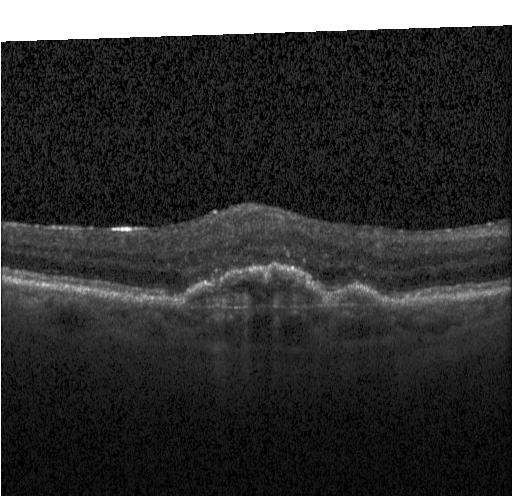

OCT scan showing choroidal neovascularization.